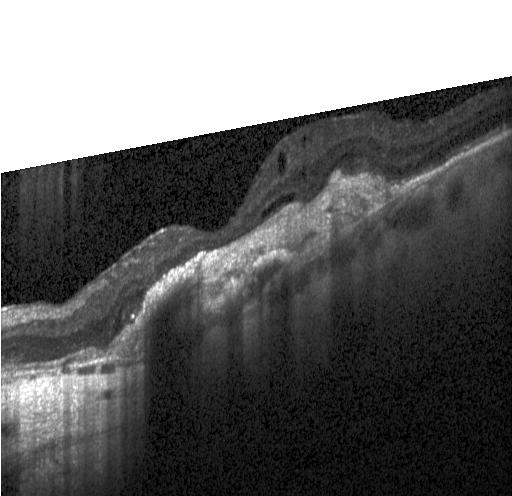

Diagnosis: choroidal neovascularization (CNV).